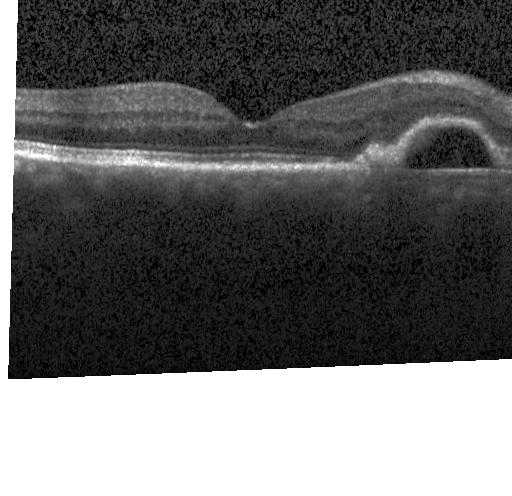
SD-OCT · optical coherence tomography B-scan · through the macula. Diagnosis: a choroidal neovascular membrane.